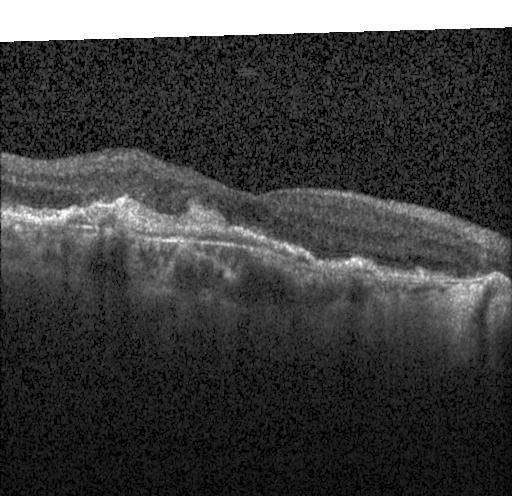
Instrument: Heidelberg Spectralis · OCT line scan — The scan shows choroidal neovascularization (CNV).